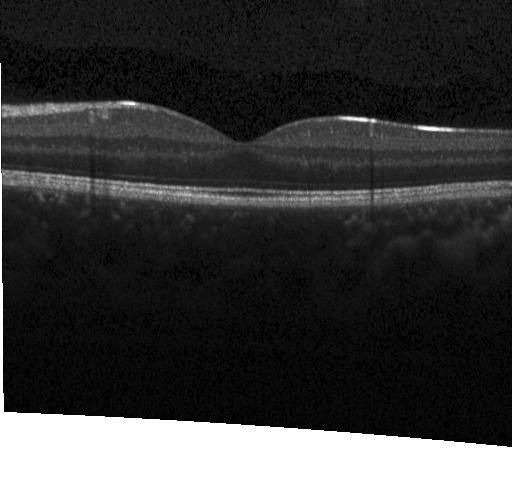 Spectral-domain optical coherence tomography, centered on the fovea, Heidelberg Spectralis, retinal OCT B-scan — Neither choroidal neovascularization, diabetic macular edema, nor drusen.